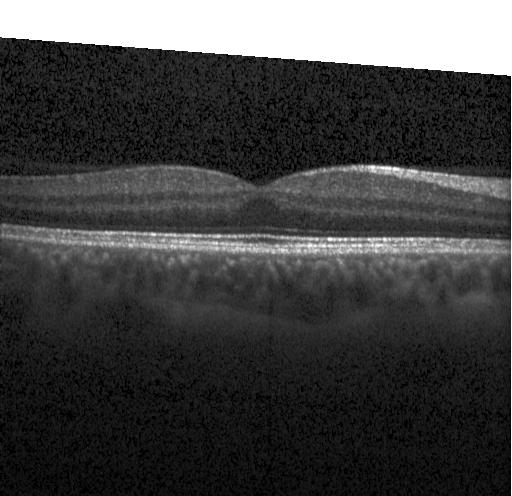

Neither choroidal neovascularization, diabetic macular edema, nor drusen.